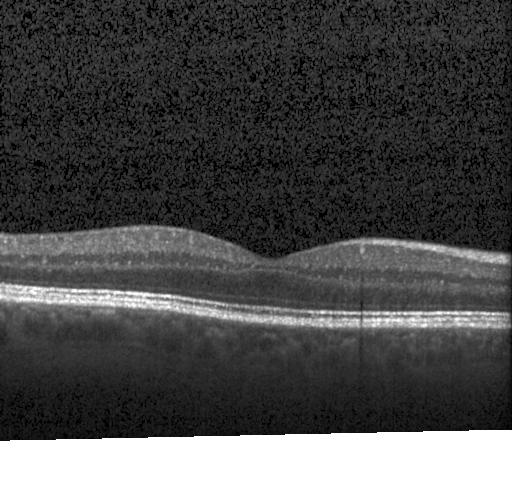 Optical coherence tomography scan, spectral-domain OCT.
No choroidal neovascularization, diabetic macular edema, or drusen.